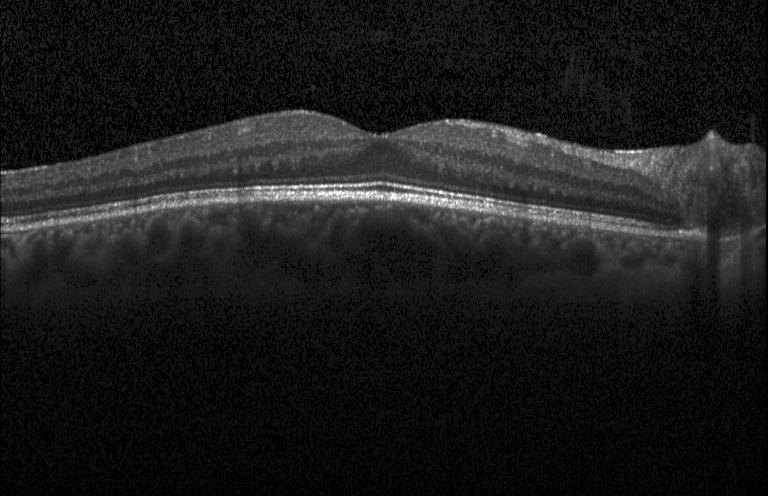 OCT B-scan
This B-scan demonstrates no CNV, DME, or drusen.